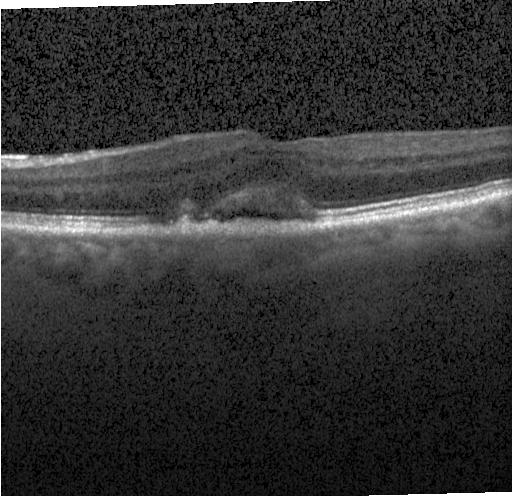
Spectral-domain OCT B-scan: choroidal neovascularization (CNV).